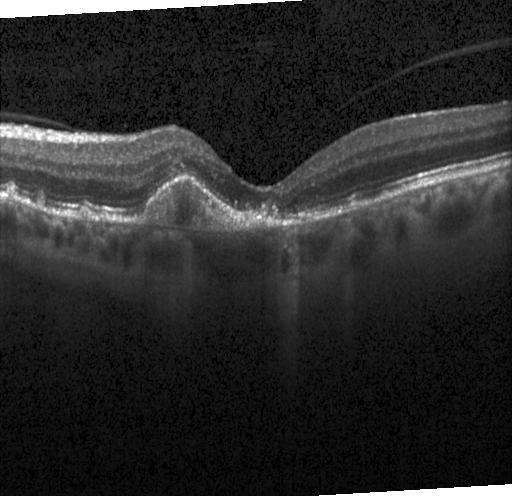 Spectral-domain optical coherence tomography · optical coherence tomography scan · Heidelberg Spectralis · centered on the fovea.
Diagnosis: choroidal neovascularization (CNV).